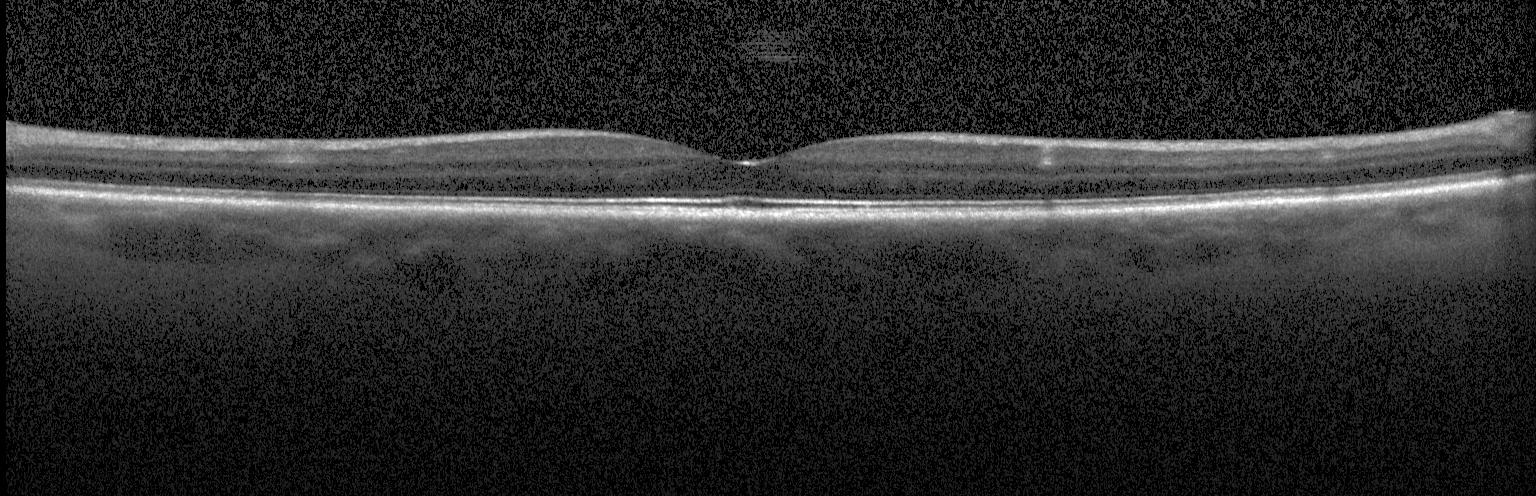 SD-OCT · acquired on a Heidelberg Spectralis · OCT line scan · horizontal scan through the fovea
Diagnosis: neither choroidal neovascularization, diabetic macular edema, nor drusen.